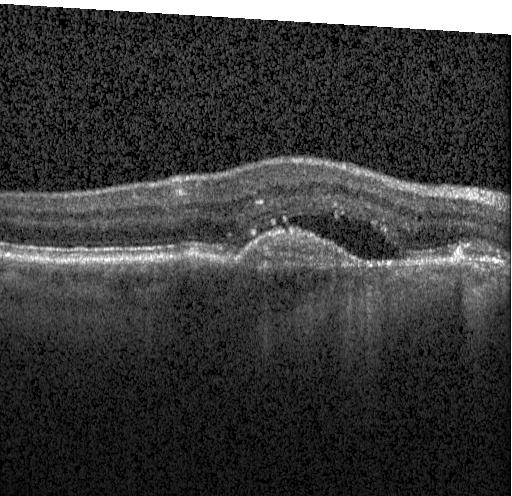 Assessment: a choroidal neovascular membrane.